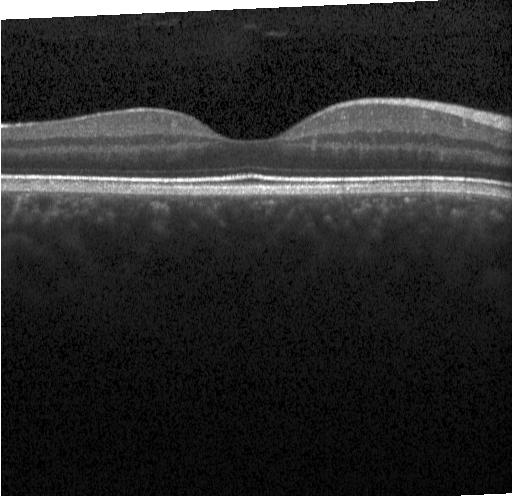
Acquired on a Heidelberg Spectralis · optical coherence tomography scan · spectral-domain OCT
Neither choroidal neovascularization, diabetic macular edema, nor drusen.